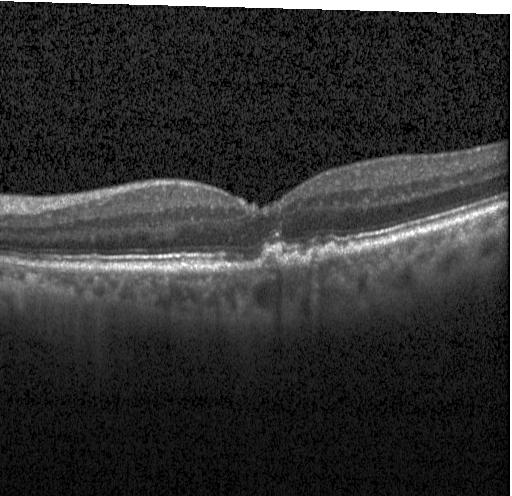
Impression: multiple drusen.